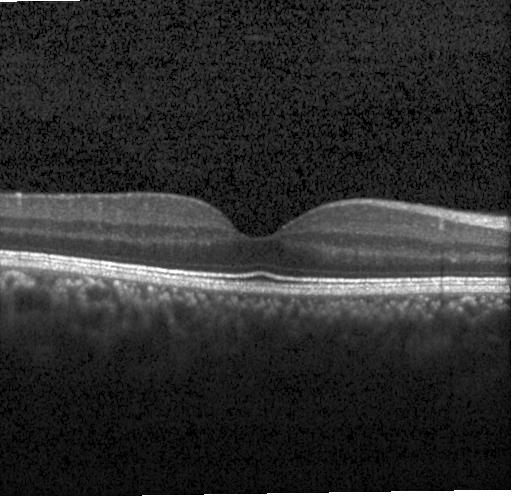
Retinal OCT B-scan, instrument: Heidelberg Spectralis
Neither choroidal neovascularization, diabetic macular edema, nor drusen.